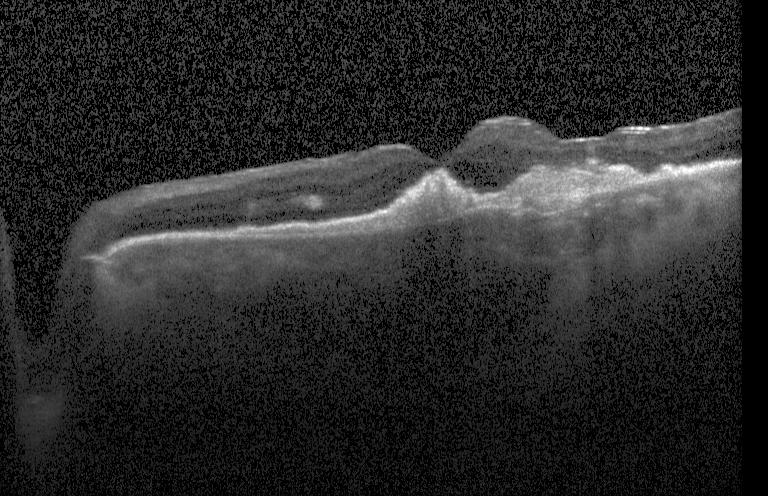
Retinal OCT cross-section, spectral-domain optical coherence tomography — OCT finding: choroidal neovascularization.